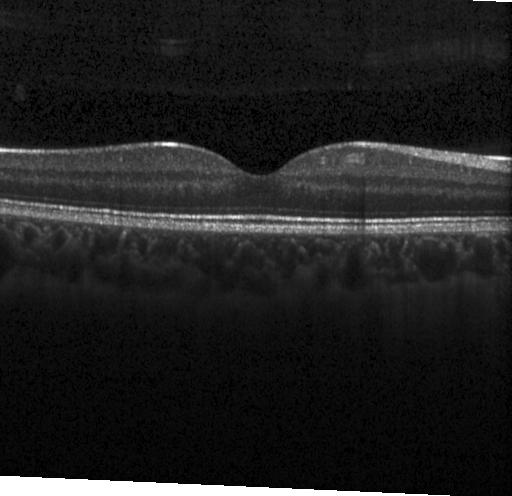
OCT B-scan, instrument: Heidelberg Spectralis.
Diagnosis: no choroidal neovascularization, no diabetic macular edema, and no drusen.